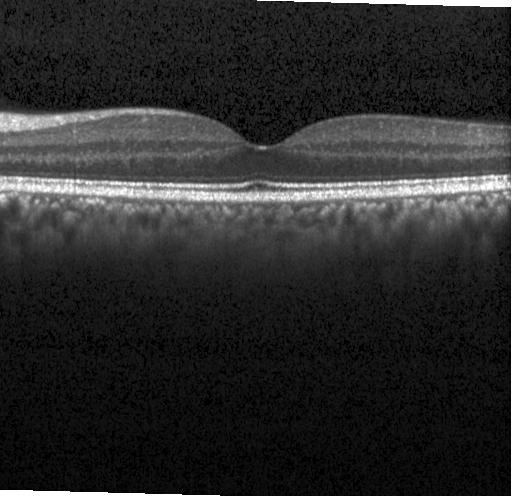
Acquired on a Heidelberg Spectralis. OCT line scan — Assessment: no evidence of CNV, DME, or drusen.